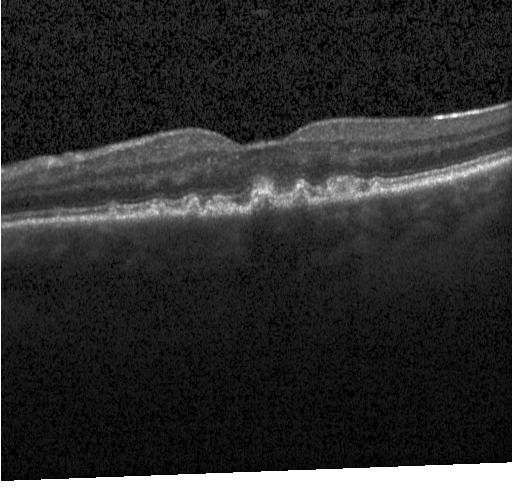
Optical coherence tomography scan. Heidelberg Spectralis OCT system. SD-OCT. Horizontal scan through the fovea. Finding: multiple drusen.